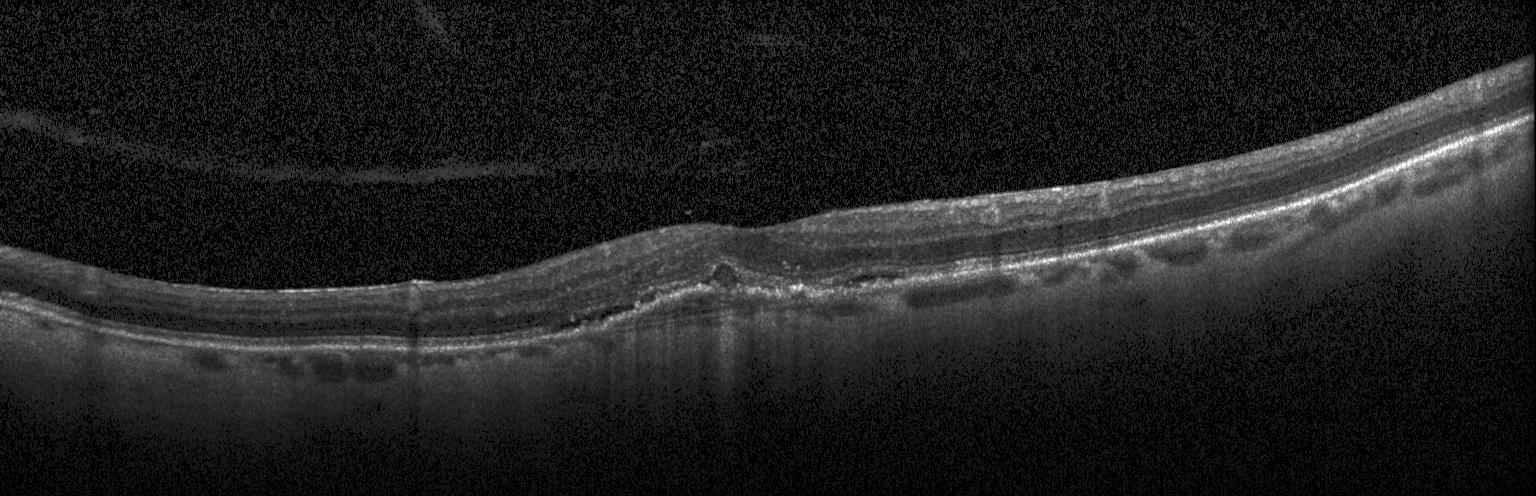
Spectral-domain OCT, retinal OCT cross-section, Heidelberg Spectralis, fovea-centered.
Diagnosis: a choroidal neovascular membrane.